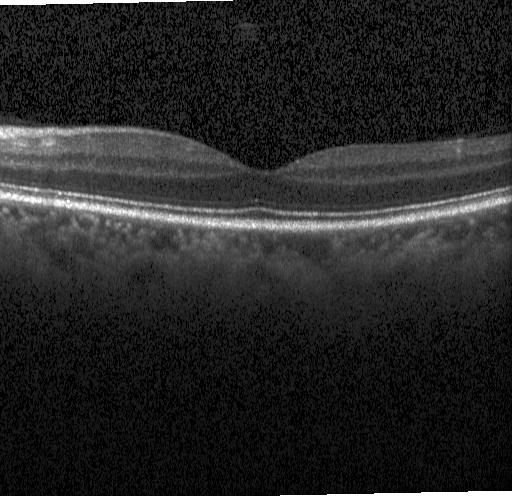
Assessment: neither choroidal neovascularization, diabetic macular edema, nor drusen.